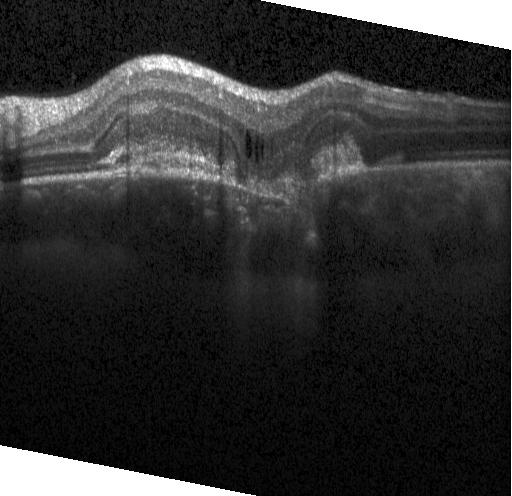

OCT B-scan — Impression: a choroidal neovascular membrane.